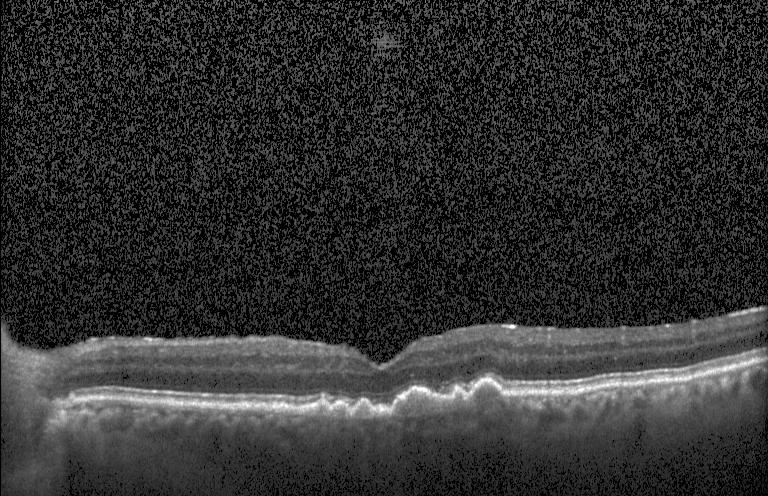 Instrument: Heidelberg Spectralis, spectral-domain optical coherence tomography, centered on the fovea, retinal OCT B-scan — Diagnosis: drusen.